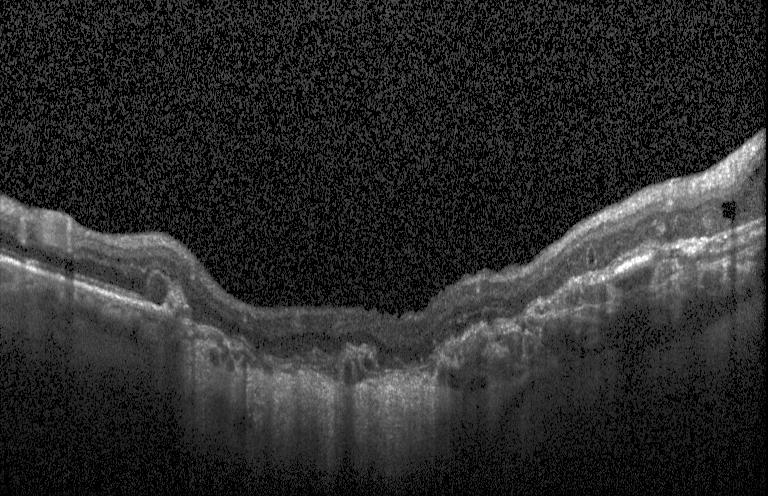
OCT B-scan.
Finding: a choroidal neovascular membrane.